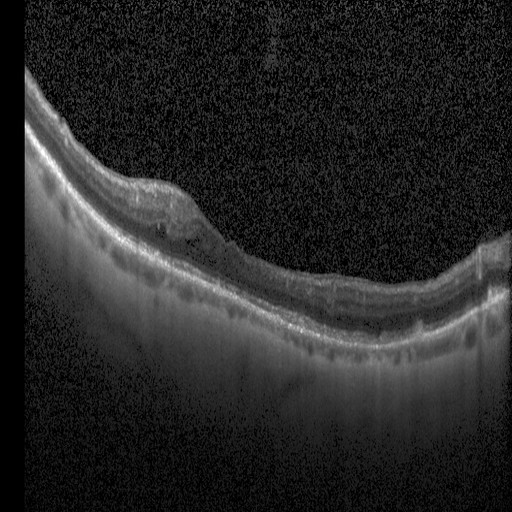
Macular OCT: diabetic macular edema (DME).